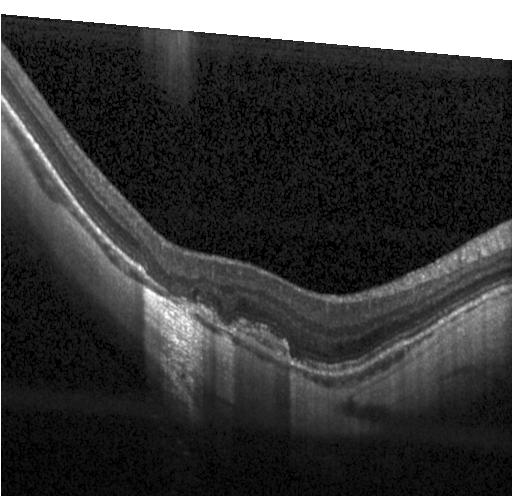

Optical coherence tomography scan — A choroidal neovascular membrane.